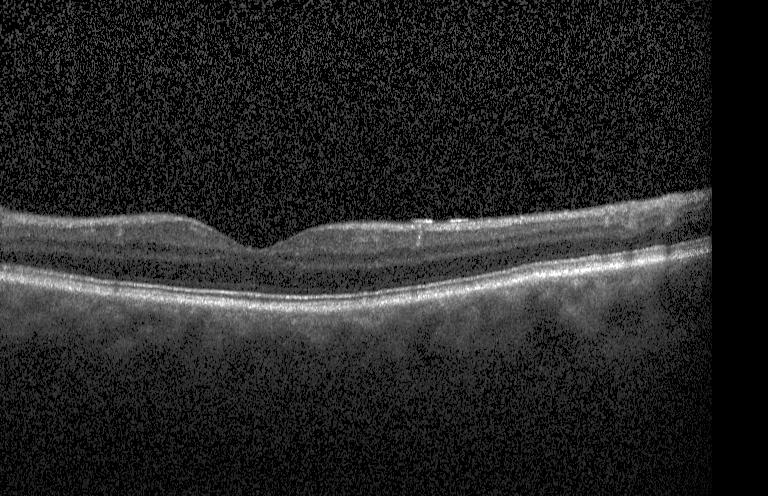

Fovea-centered; retinal OCT B-scan; SD-OCT.
Neither CNV, DME, nor drusen.